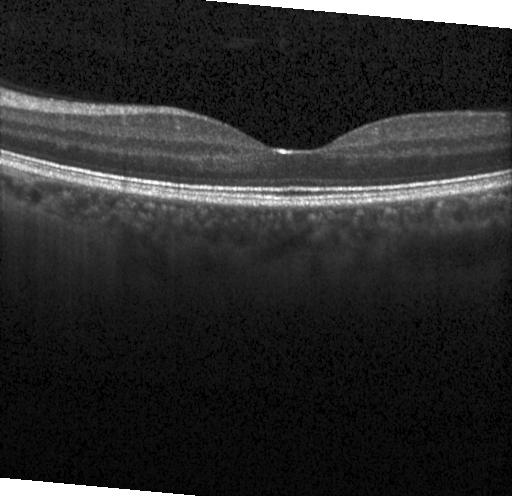
Spectral-domain optical coherence tomography; macular scan; optical coherence tomography B-scan; Heidelberg Spectralis.
Diagnosis: no choroidal neovascularization, no diabetic macular edema, and no drusen.